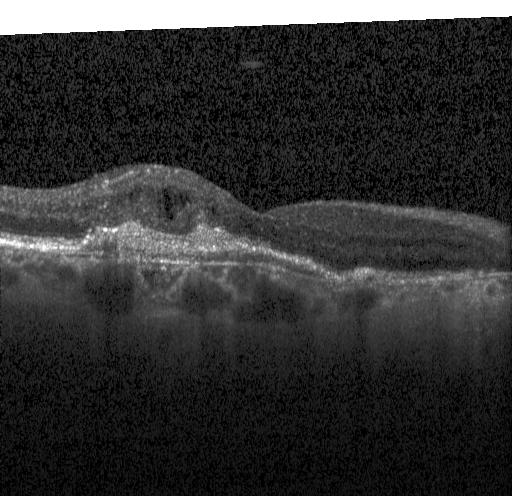
SD-OCT; retinal OCT cross-section. OCT finding: choroidal neovascularization.